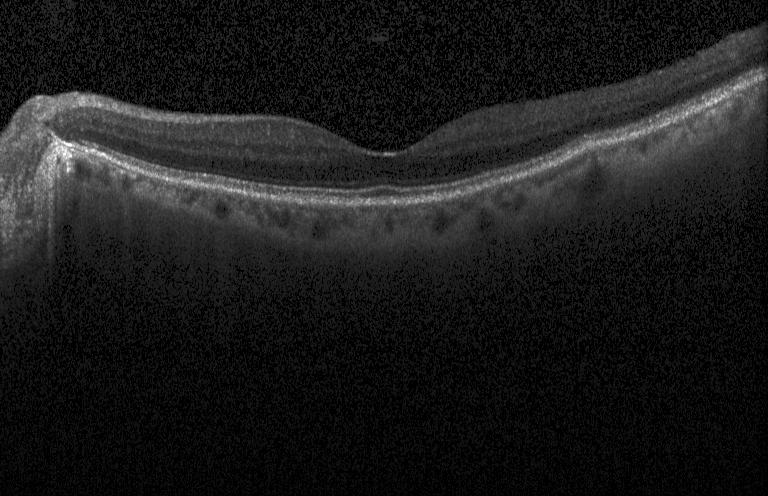
Dx: no evidence of choroidal neovascularization, diabetic macular edema, or drusen.